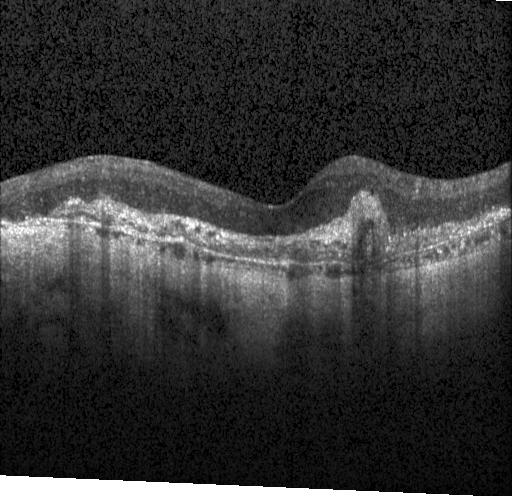 Heidelberg Spectralis. OCT line scan. SD-OCT. Through the macula
Finding: choroidal neovascularization.